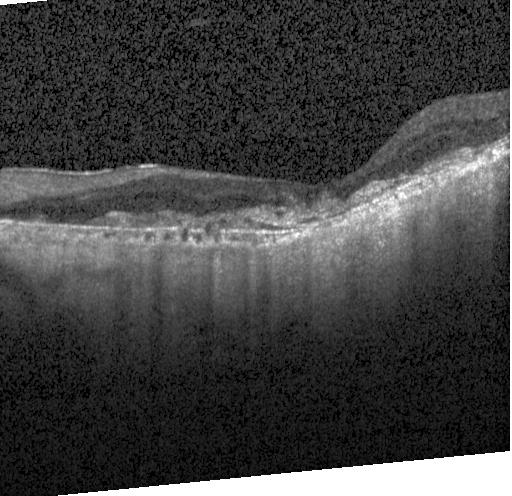

Retinal OCT B-scan.
Dx: a choroidal neovascular membrane.